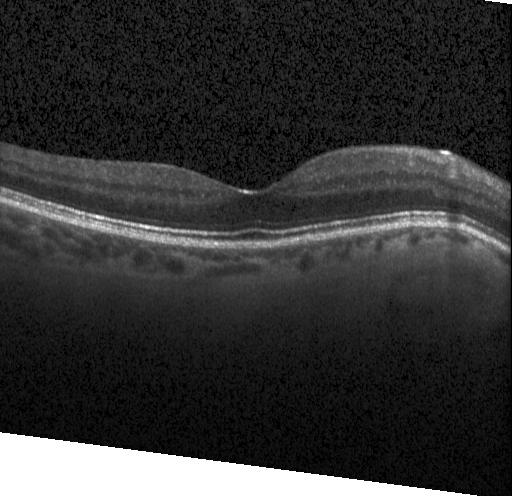 Spectral-domain OCT B-scan: no choroidal neovascularization, no diabetic macular edema, and no drusen.